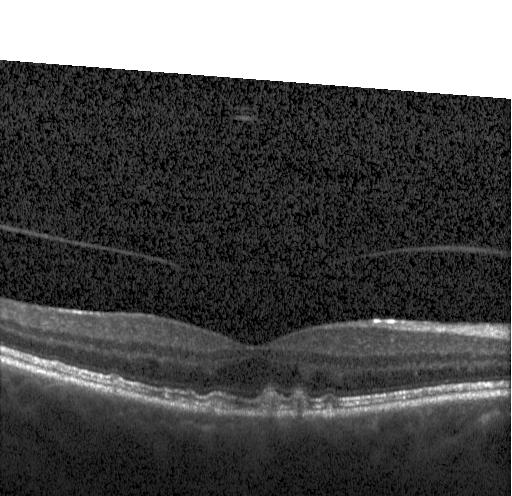 Instrument: Heidelberg Spectralis · OCT line scan · spectral-domain optical coherence tomography.
Finding: sub-RPE drusenoid deposits.